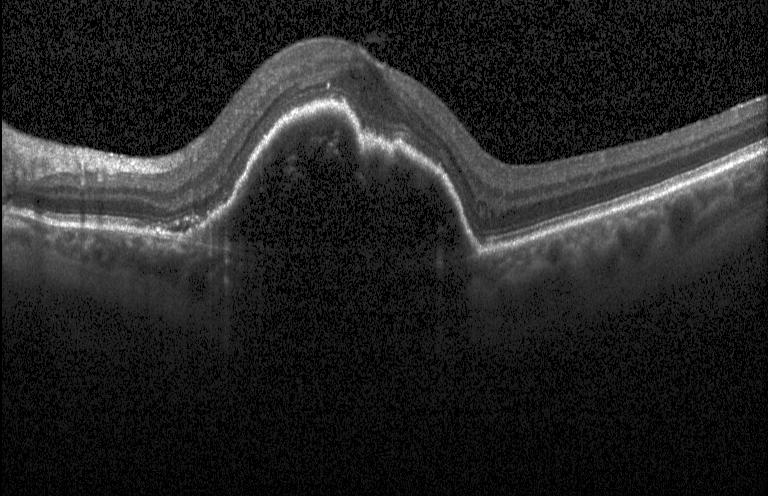

OCT B-scan
OCT finding: CNV.